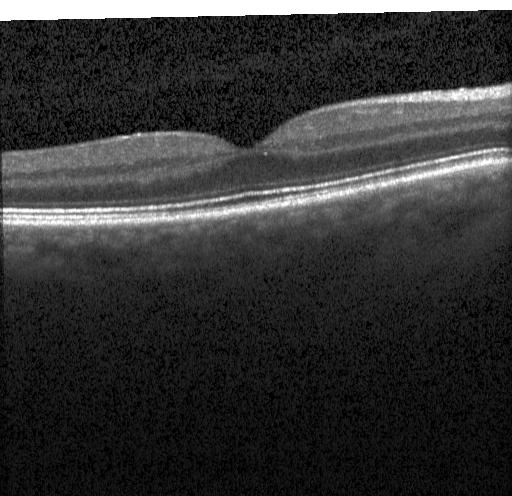

Macular scan · optical coherence tomography scan
This B-scan demonstrates no choroidal neovascularization, diabetic macular edema, or drusen.